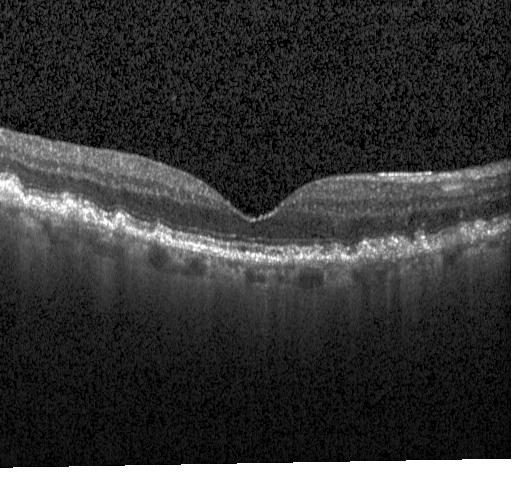

Macular OCT demonstrating sub-RPE drusenoid deposits.